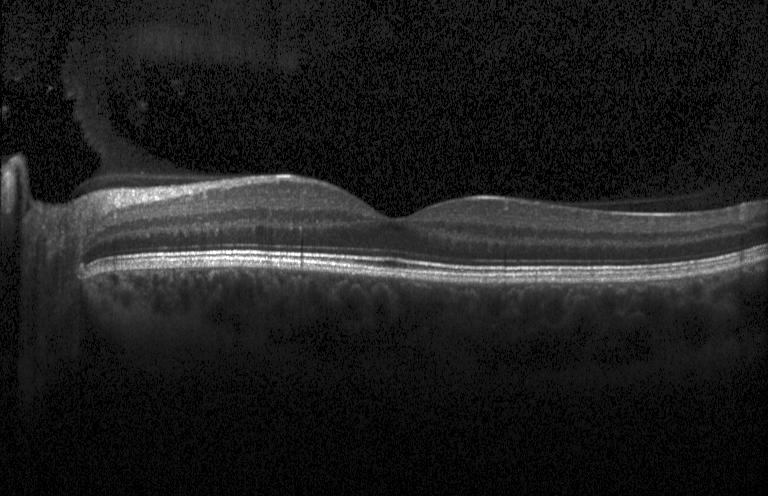 OCT line scan. The scan shows no choroidal neovascularization, no diabetic macular edema, and no drusen.